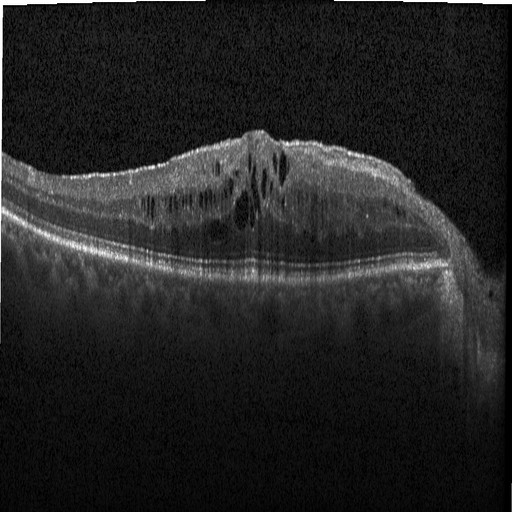 OCT scan showing DME.